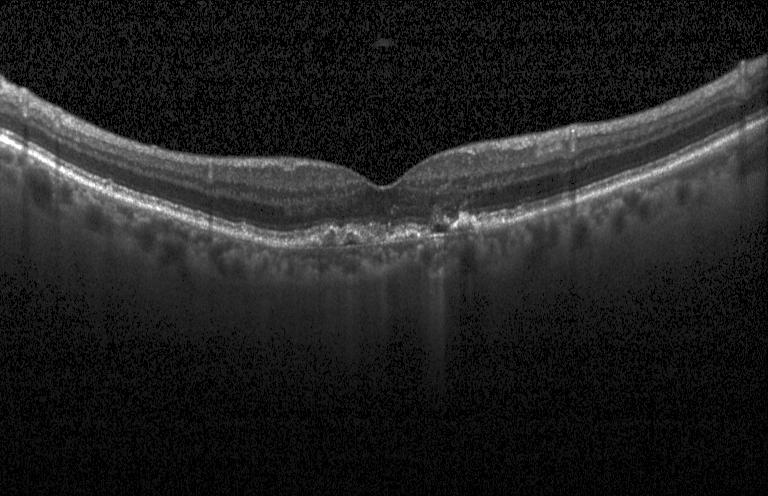
SD-OCT; OCT line scan.
Choroidal neovascularization.